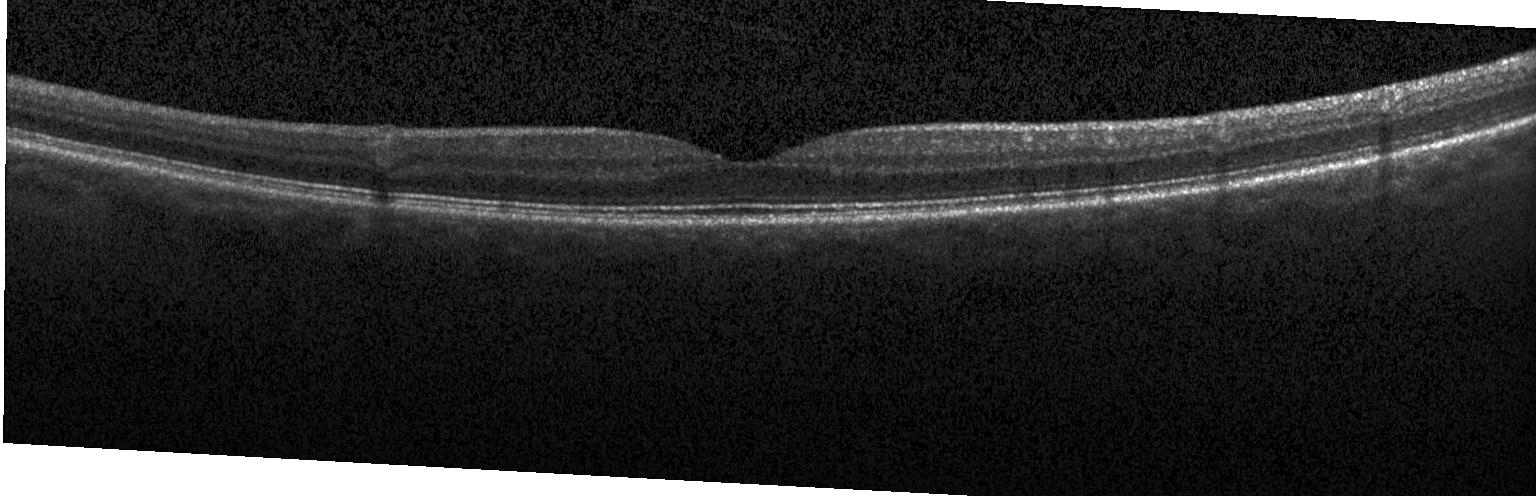
Macular OCT: no choroidal neovascularization, diabetic macular edema, or drusen.